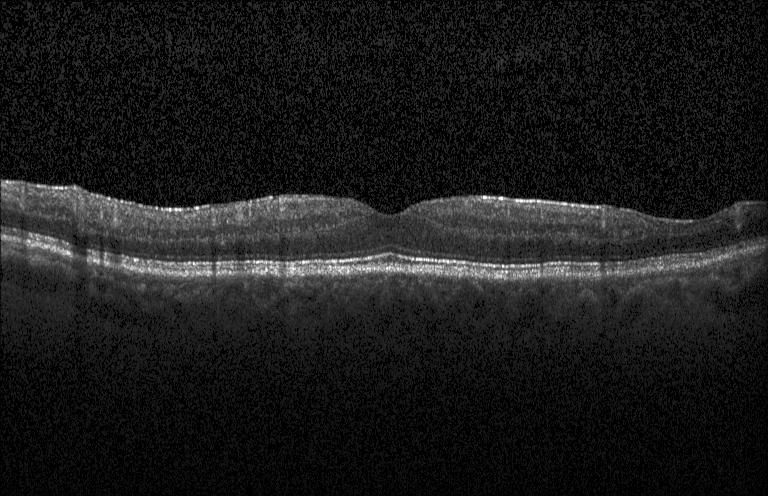

SD-OCT · horizontal scan through the fovea · retinal OCT cross-section — Macular OCT: no evidence of choroidal neovascularization, diabetic macular edema, or drusen.